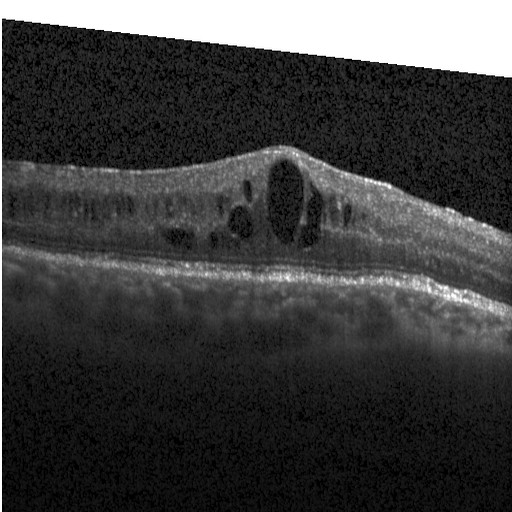
Dx: DME.